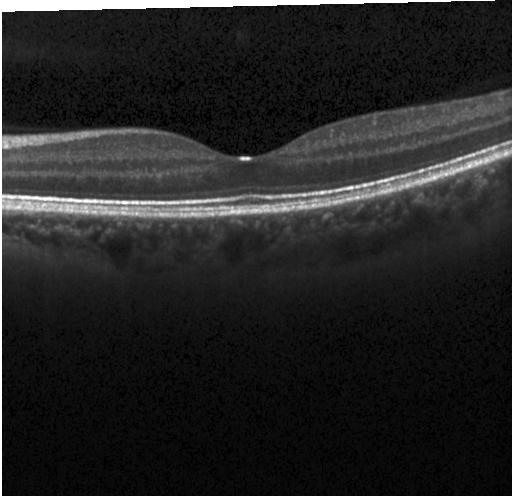 OCT B-scan
Finding: no evidence of choroidal neovascularization, diabetic macular edema, or drusen.